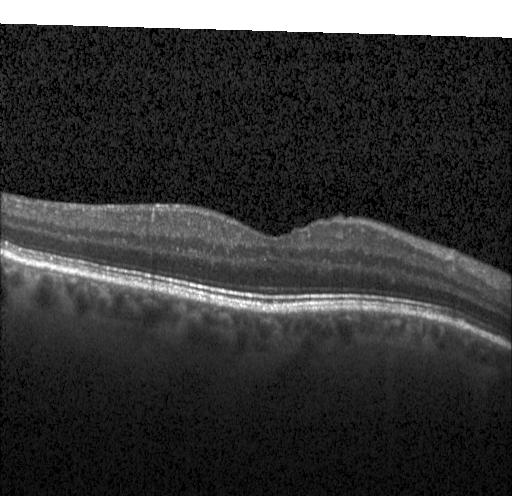
Finding: no CNV, DME, or drusen.